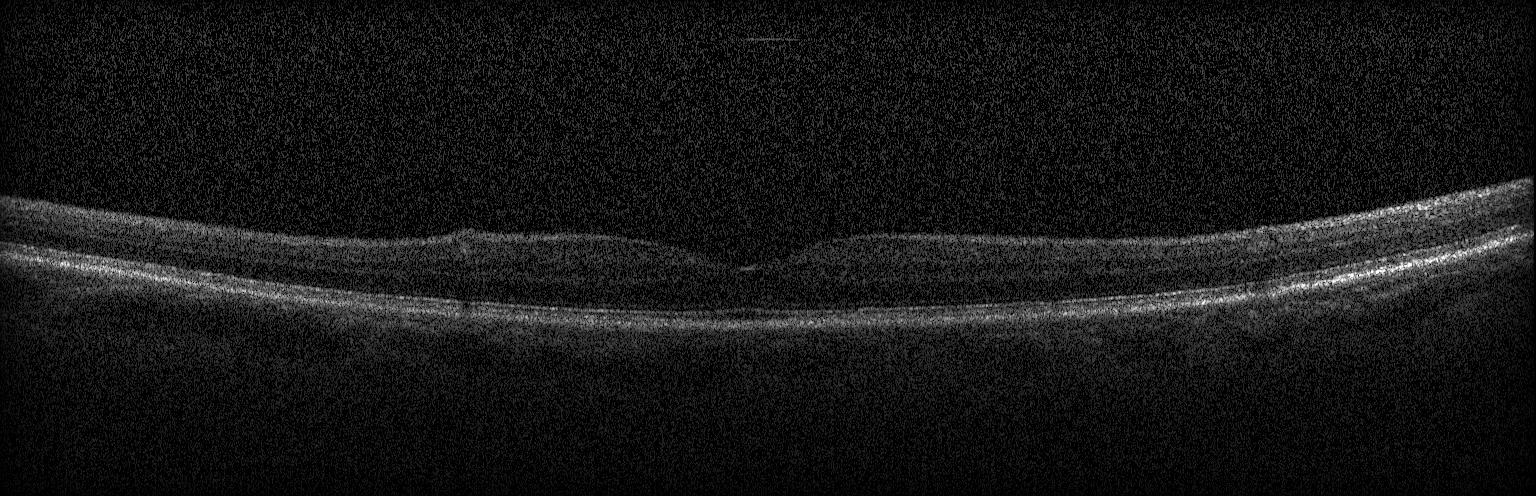

Fovea-centered. Retinal OCT B-scan. Spectral-domain OCT.
Dx: no choroidal neovascularization, no diabetic macular edema, and no drusen.